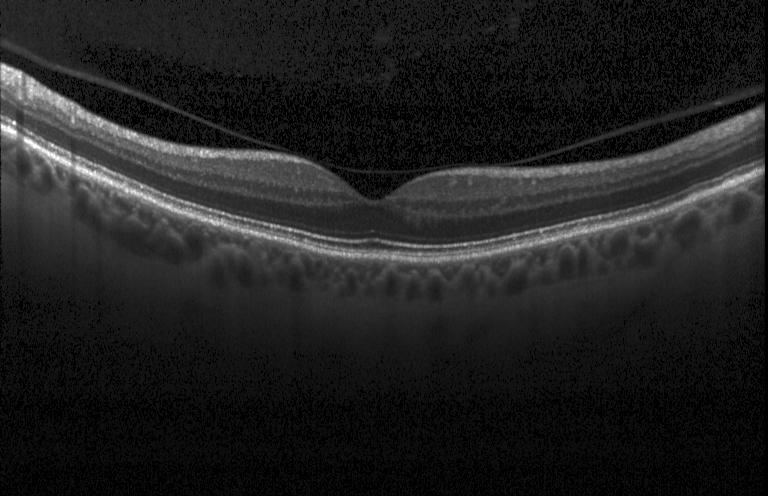 OCT B-scan · instrument: Heidelberg Spectralis. Impression: neither choroidal neovascularization, diabetic macular edema, nor drusen.